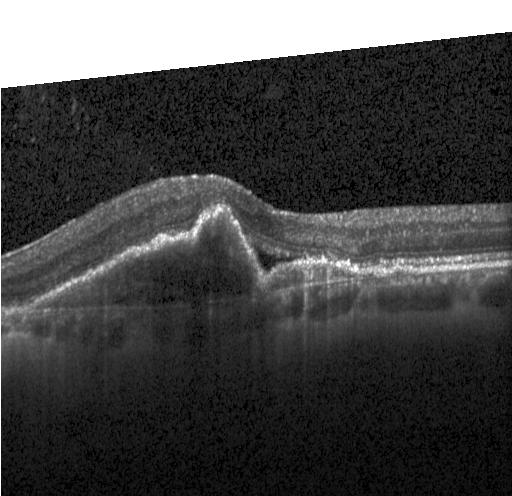
OCT B-scan.
This B-scan demonstrates choroidal neovascularization (CNV).